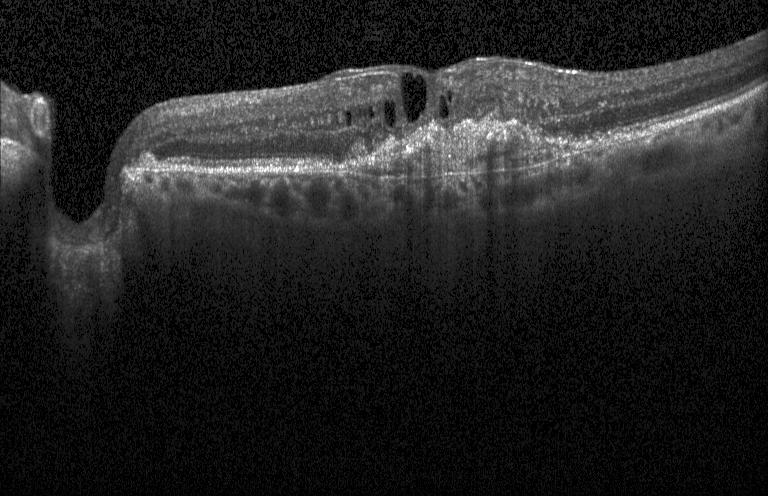
OCT line scan
Diagnosis: a choroidal neovascular membrane.